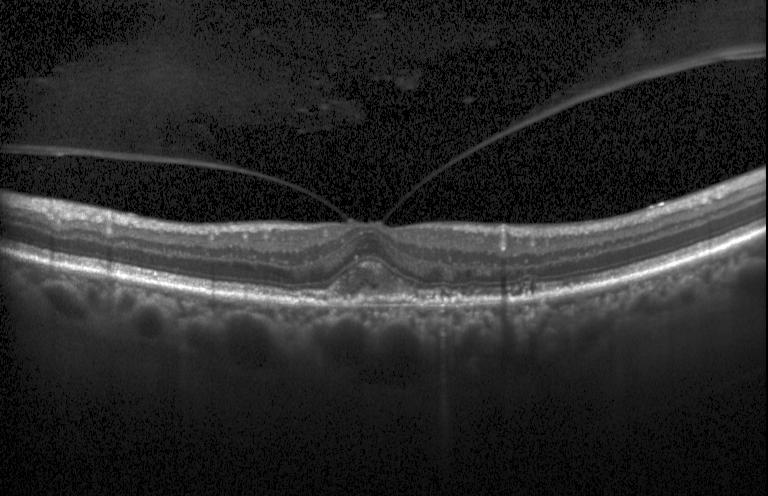 Diagnosis: CNV.